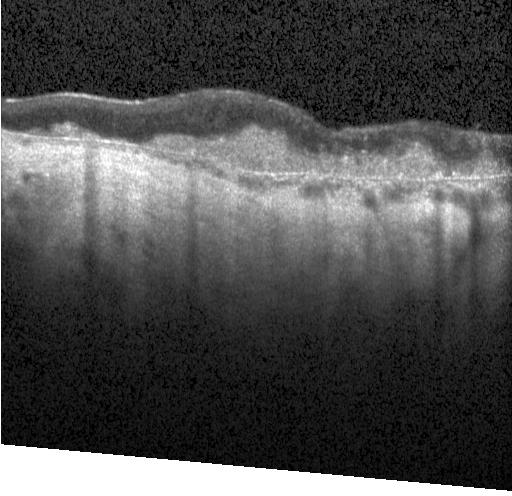
Centered on the fovea · OCT line scan
Macular OCT: CNV.